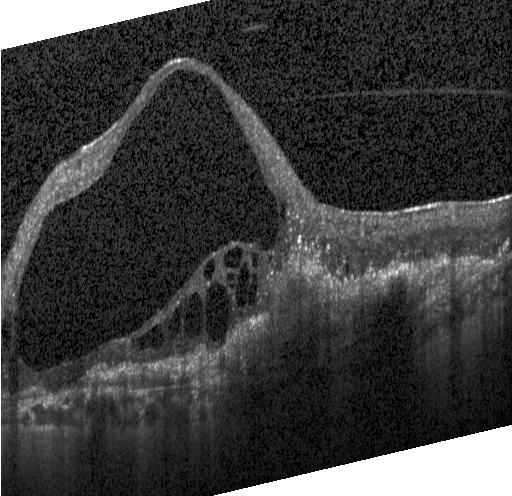 Optical coherence tomography B-scan — Macular OCT: choroidal neovascularization (CNV).